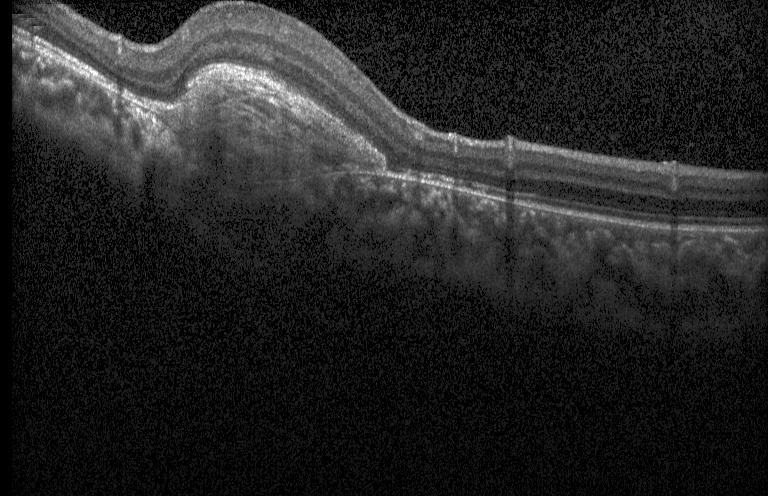

OCT line scan. Through the macula. Heidelberg Spectralis. Spectral-domain optical coherence tomography
Impression: a choroidal neovascular membrane.